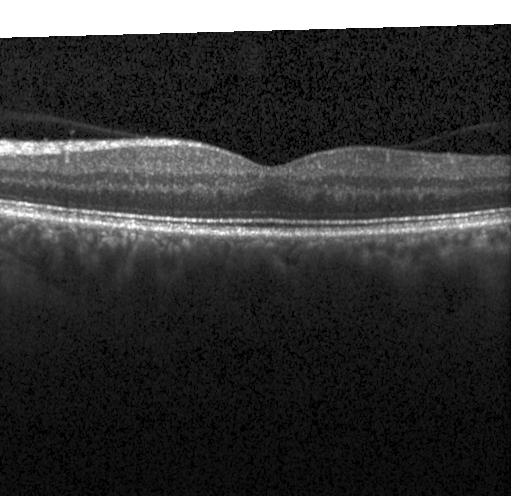
OCT line scan
Assessment: neither choroidal neovascularization, diabetic macular edema, nor drusen.